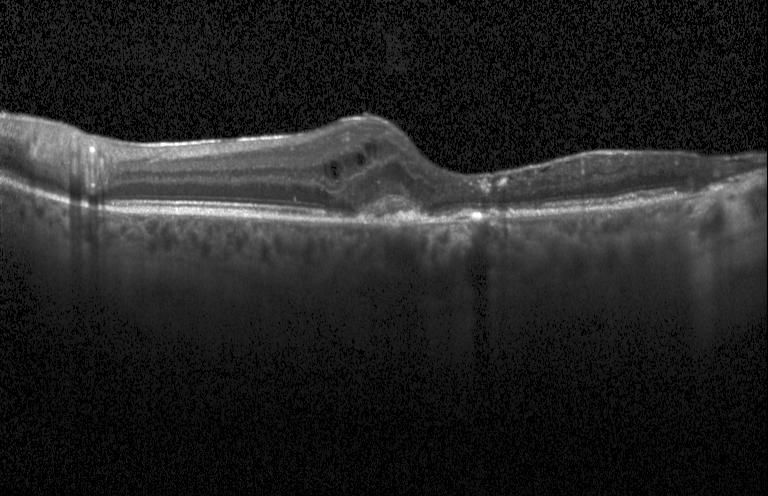

Spectral-domain optical coherence tomography; retinal OCT cross-section; Heidelberg Spectralis OCT system; through the macula. Dx: choroidal neovascularization (CNV).